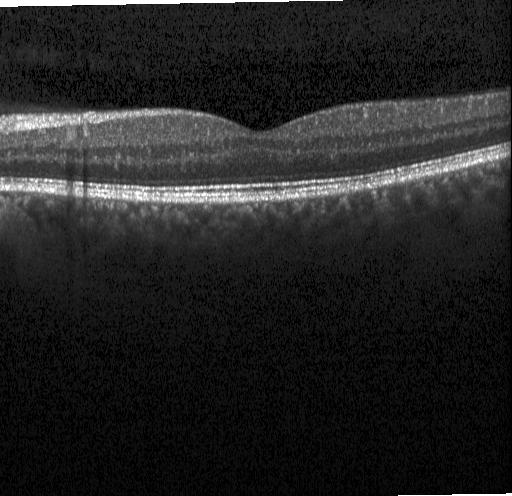
Finding: neither CNV, DME, nor drusen.